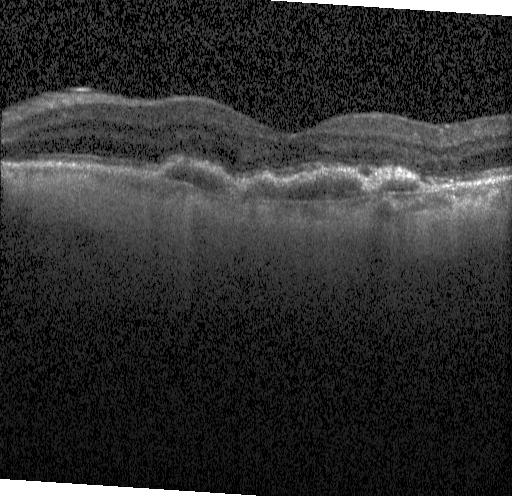
Diagnosis: a choroidal neovascular membrane.